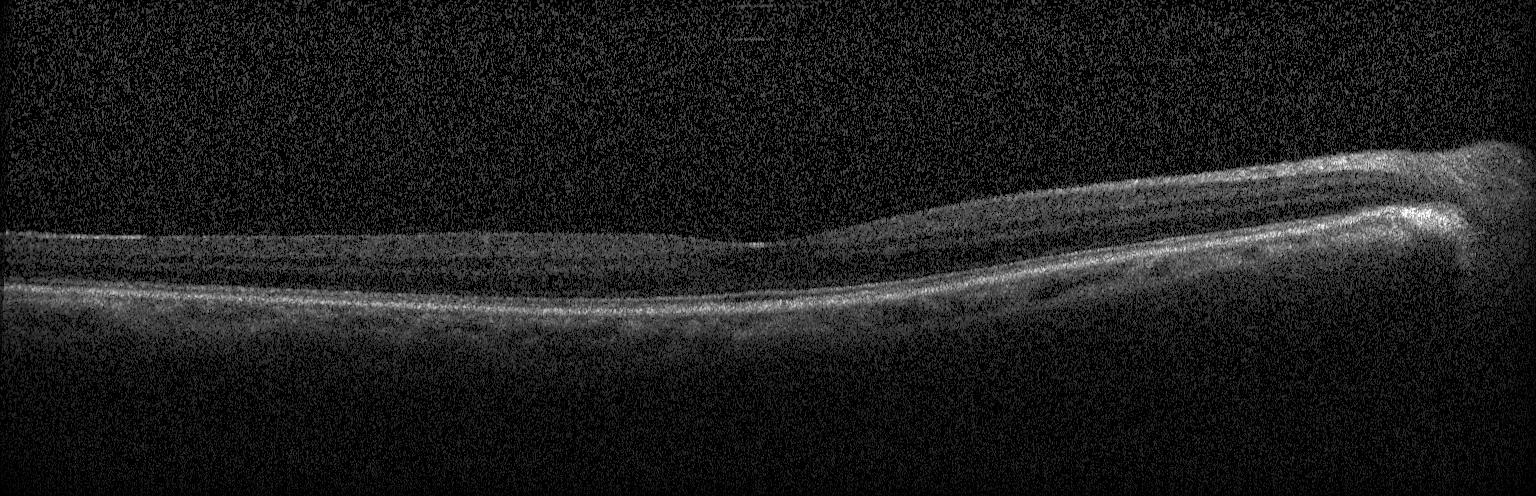
Centered on the fovea; Heidelberg Spectralis; spectral-domain OCT; optical coherence tomography scan
Dx: no choroidal neovascularization, no diabetic macular edema, and no drusen.